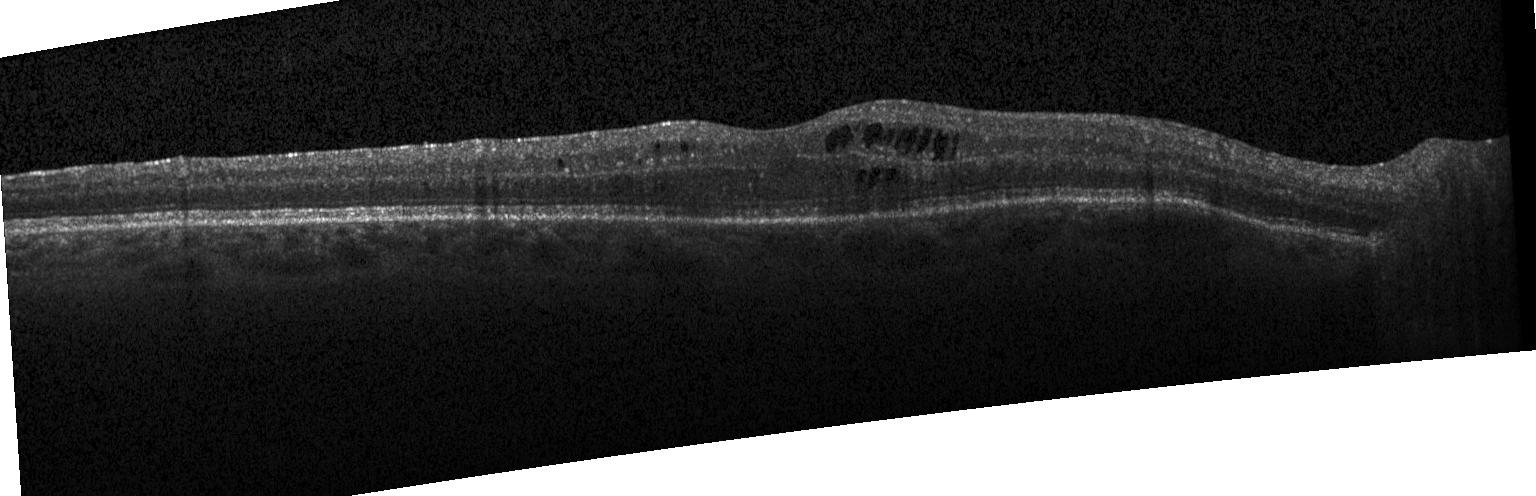
Spectral-domain OCT, retinal OCT B-scan, instrument: Heidelberg Spectralis, through the macula — Assessment: diabetic macular edema (DME).